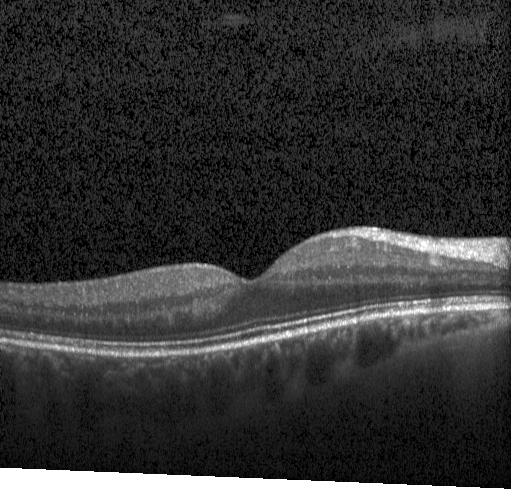 OCT line scan · horizontal scan through the fovea
Diagnosis: no choroidal neovascularization, no diabetic macular edema, and no drusen.